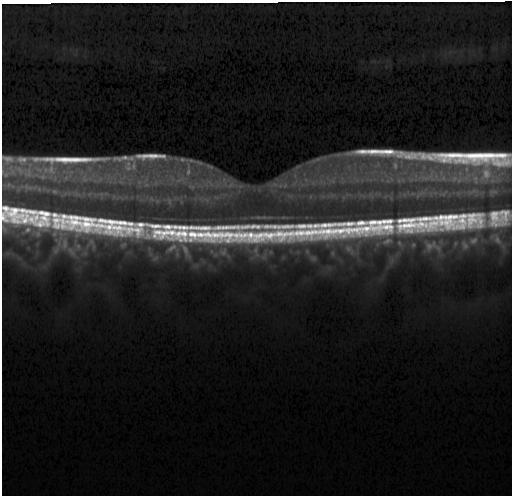
SD-OCT · retinal OCT cross-section.
No evidence of choroidal neovascularization, diabetic macular edema, or drusen.